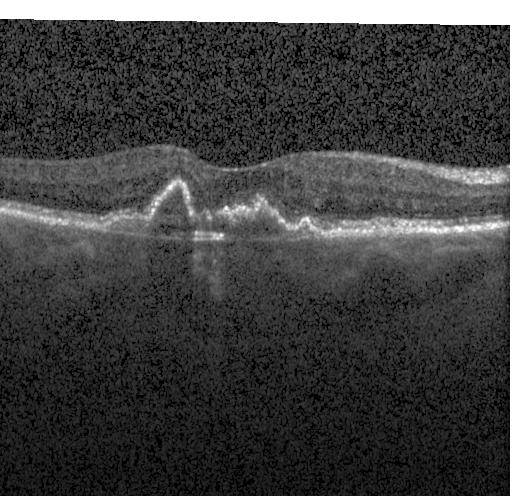 Dx: a choroidal neovascular membrane.